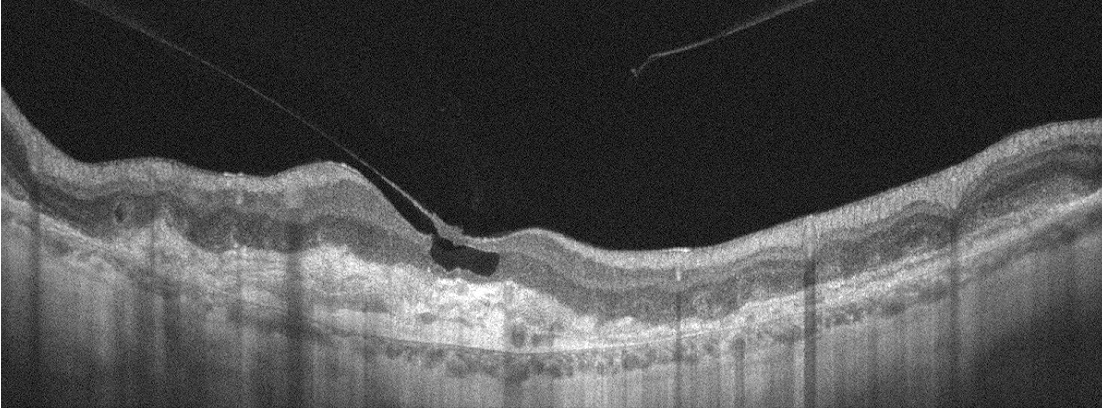 Macular OCT: age-related macular degeneration (AMD).